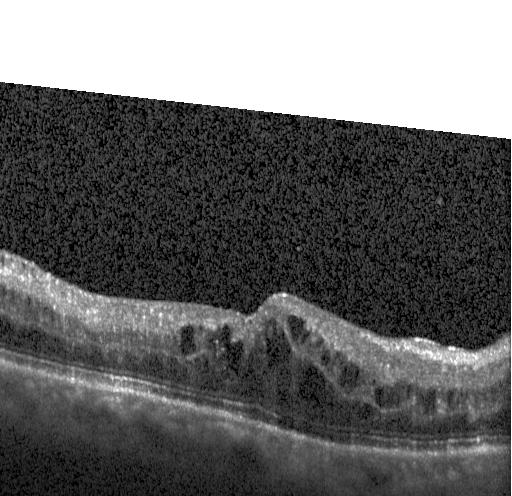 Optical coherence tomography B-scan · spectral-domain OCT · Heidelberg Spectralis OCT system
Dx: DME.